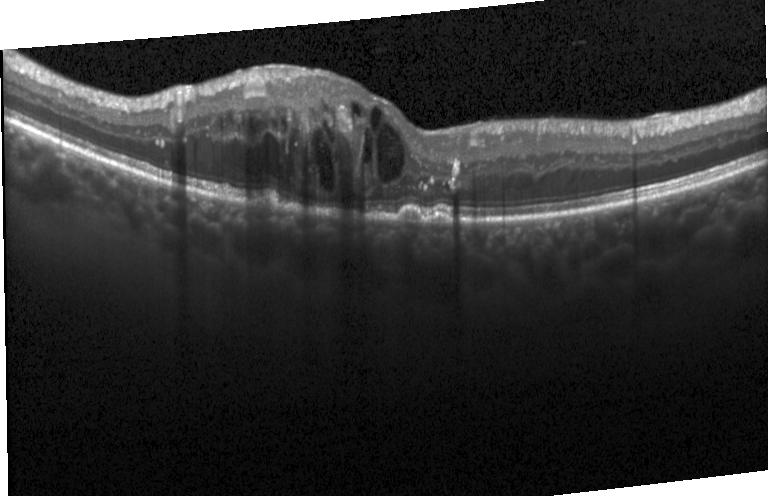 Optical coherence tomography scan, spectral-domain optical coherence tomography, horizontal scan through the fovea.
Finding: DME.